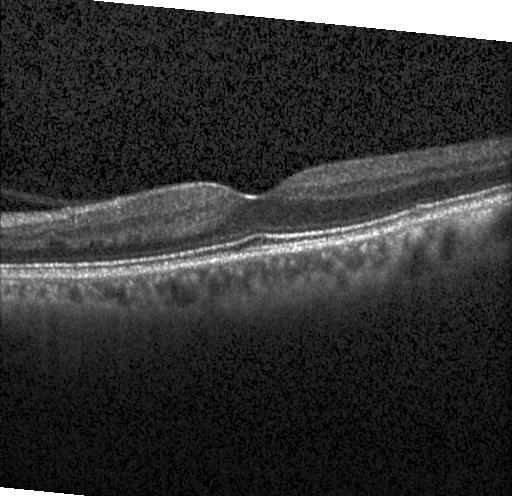 Diagnosis: no choroidal neovascularization, diabetic macular edema, or drusen.